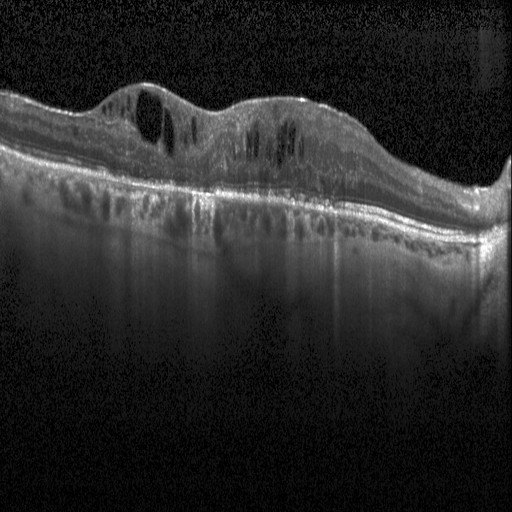 Instrument: Heidelberg Spectralis · optical coherence tomography scan · fovea-centered. The scan shows diabetic macular edema (DME).